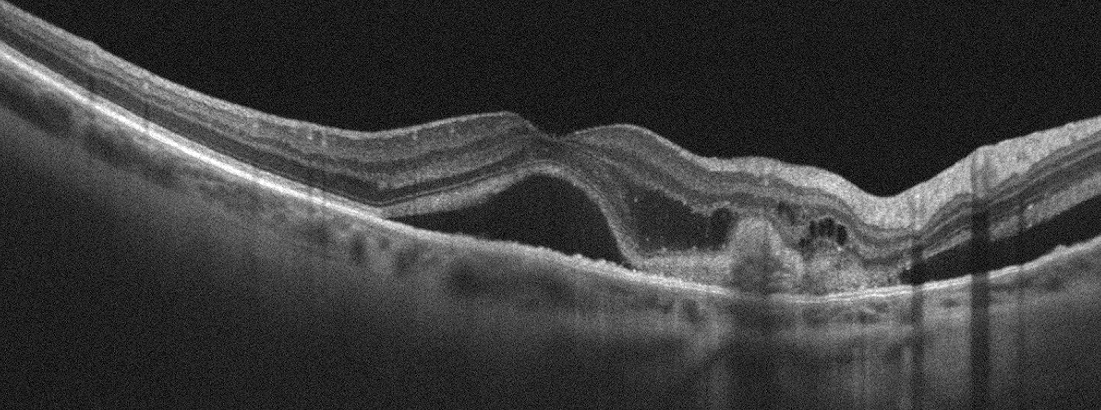
Optical coherence tomography B-scan — Finding: age-related macular degeneration (AMD).